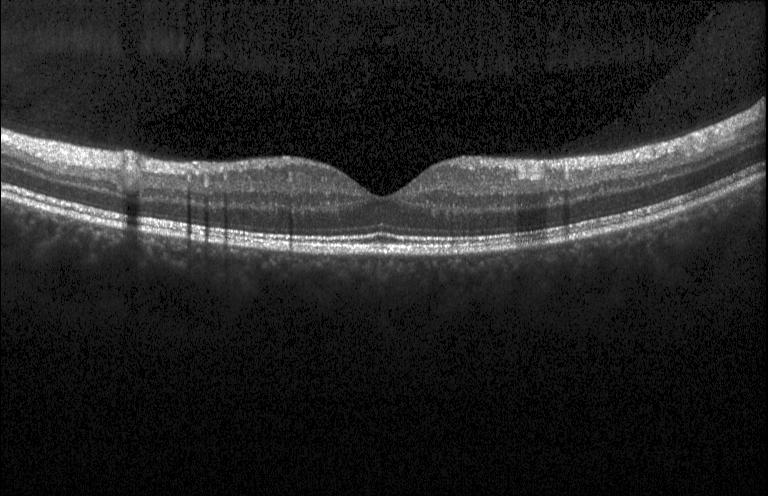

Horizontal scan through the fovea · OCT line scan.
Dx: no choroidal neovascularization, diabetic macular edema, or drusen.